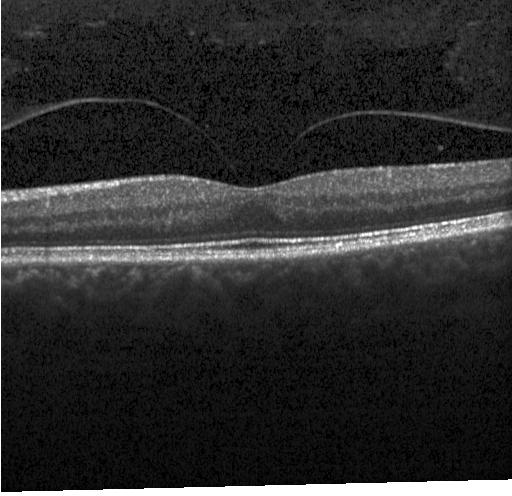
Optical coherence tomography scan · centered on the fovea · SD-OCT · instrument: Heidelberg Spectralis.
Macular OCT: no choroidal neovascularization, diabetic macular edema, or drusen.